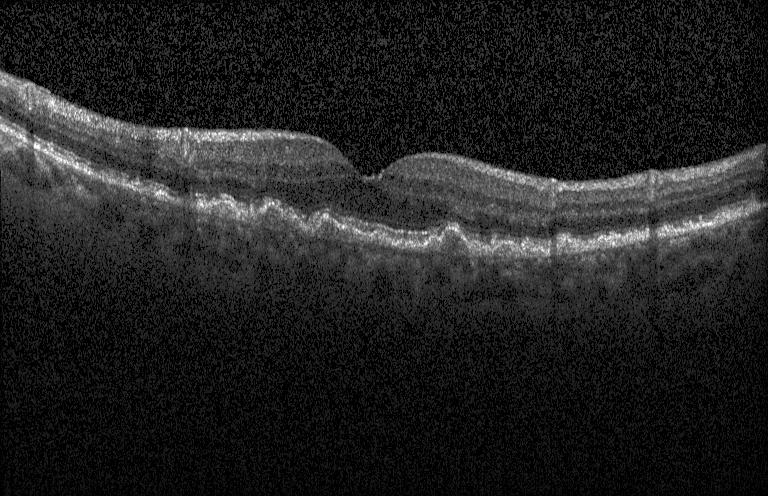 Through the macula, optical coherence tomography B-scan, Heidelberg Spectralis OCT system, SD-OCT. Impression: drusen.